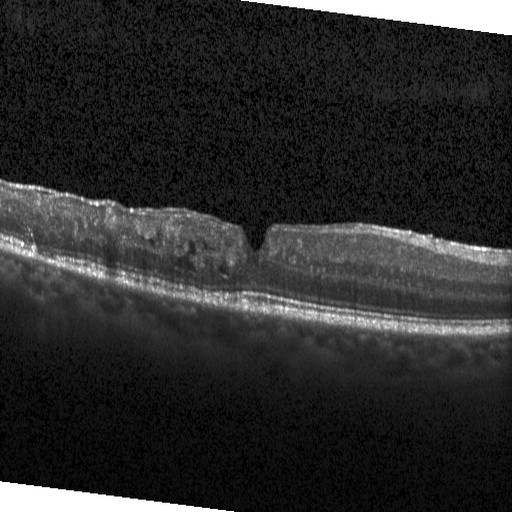
Retinal OCT cross-section
Macular OCT: DME.